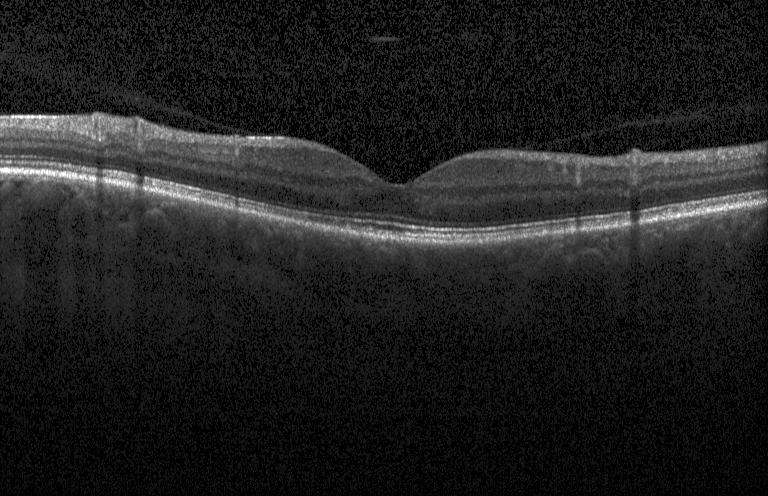
Centered on the fovea, retinal OCT cross-section. The scan shows no choroidal neovascularization, diabetic macular edema, or drusen.